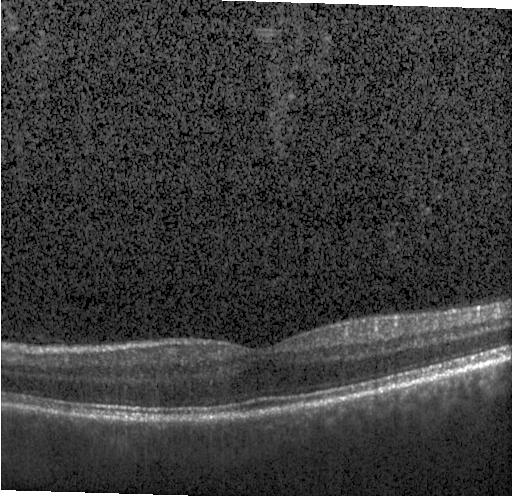
Through the macula · retinal OCT cross-section · spectral-domain OCT. Dx: no choroidal neovascularization, diabetic macular edema, or drusen.